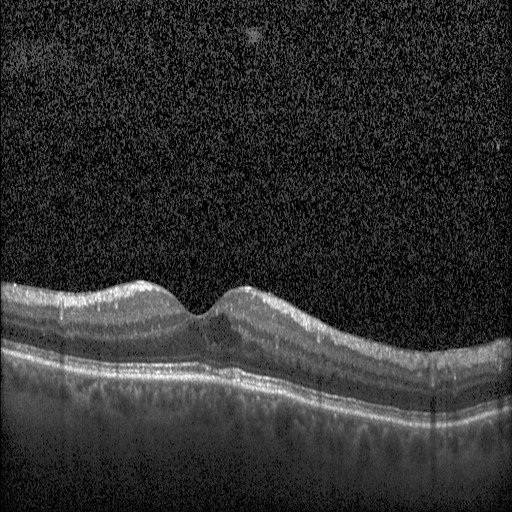
Spectral-domain OCT. Optical coherence tomography B-scan. Fovea-centered.
OCT finding: diabetic macular edema.